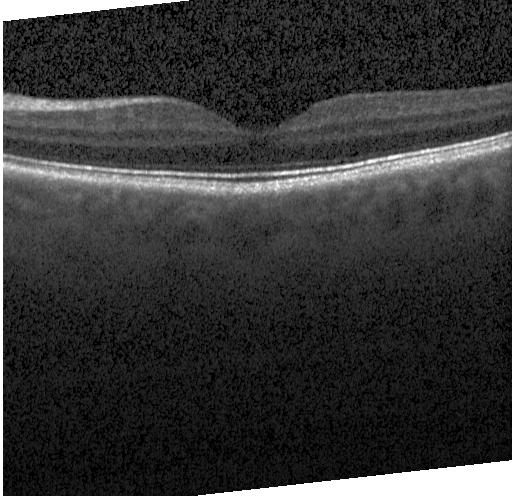

Retinal OCT B-scan. Fovea-centered — No choroidal neovascularization, no diabetic macular edema, and no drusen.